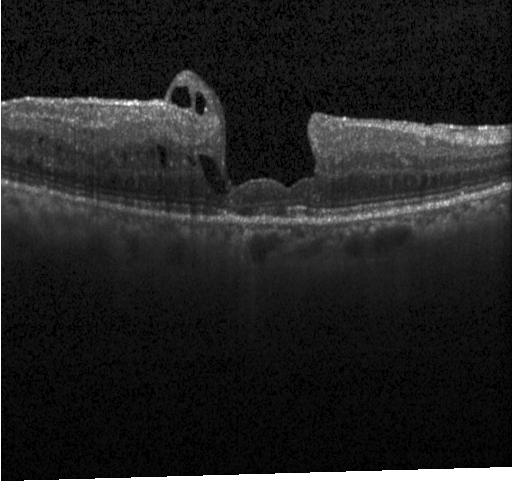
OCT B-scan — The scan shows DME.